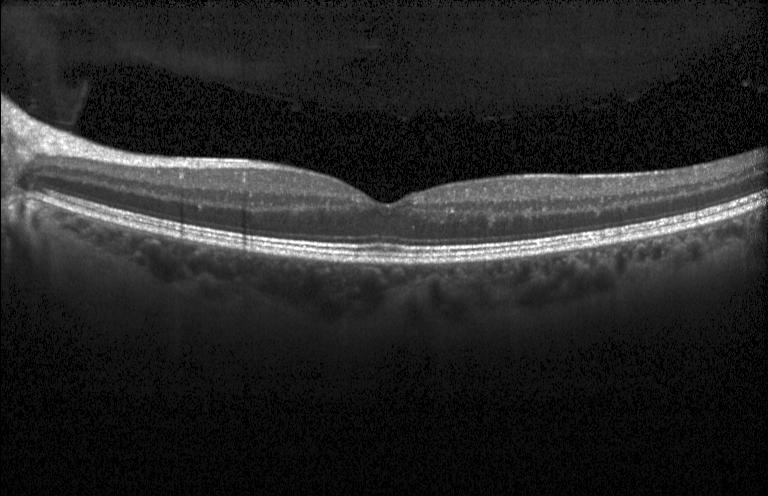

Heidelberg Spectralis · optical coherence tomography B-scan — Impression: no choroidal neovascularization, diabetic macular edema, or drusen.